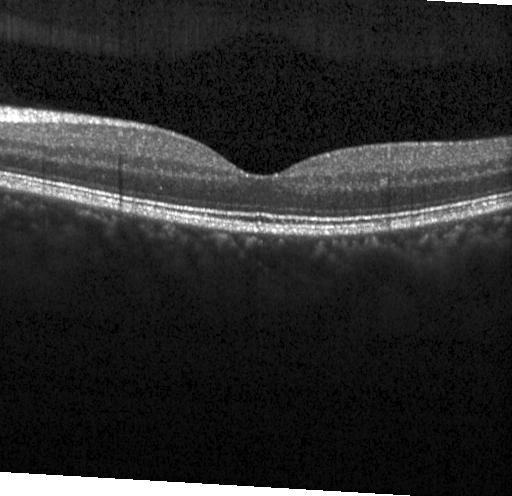
Spectral-domain OCT B-scan: no choroidal neovascularization, no diabetic macular edema, and no drusen.